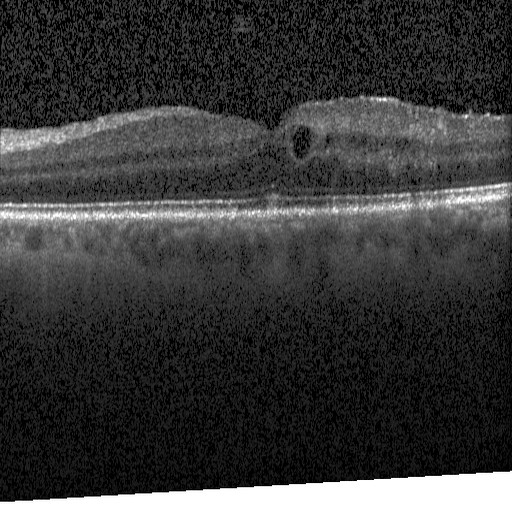
Diabetic macular edema (DME).